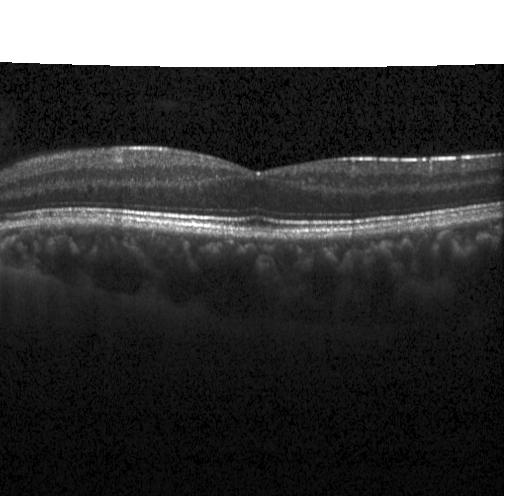
Retinal OCT B-scan
No choroidal neovascularization, diabetic macular edema, or drusen.